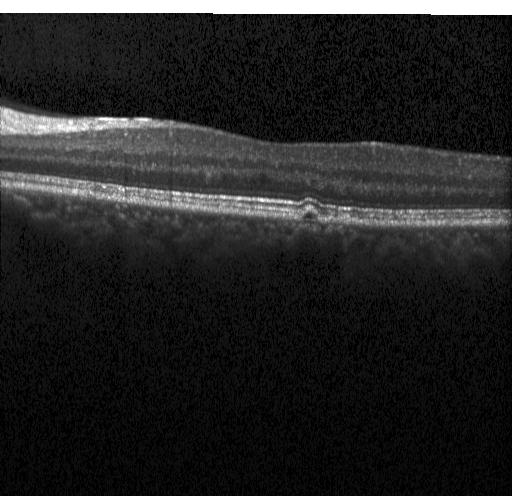
OCT finding: sub-RPE drusenoid deposits.